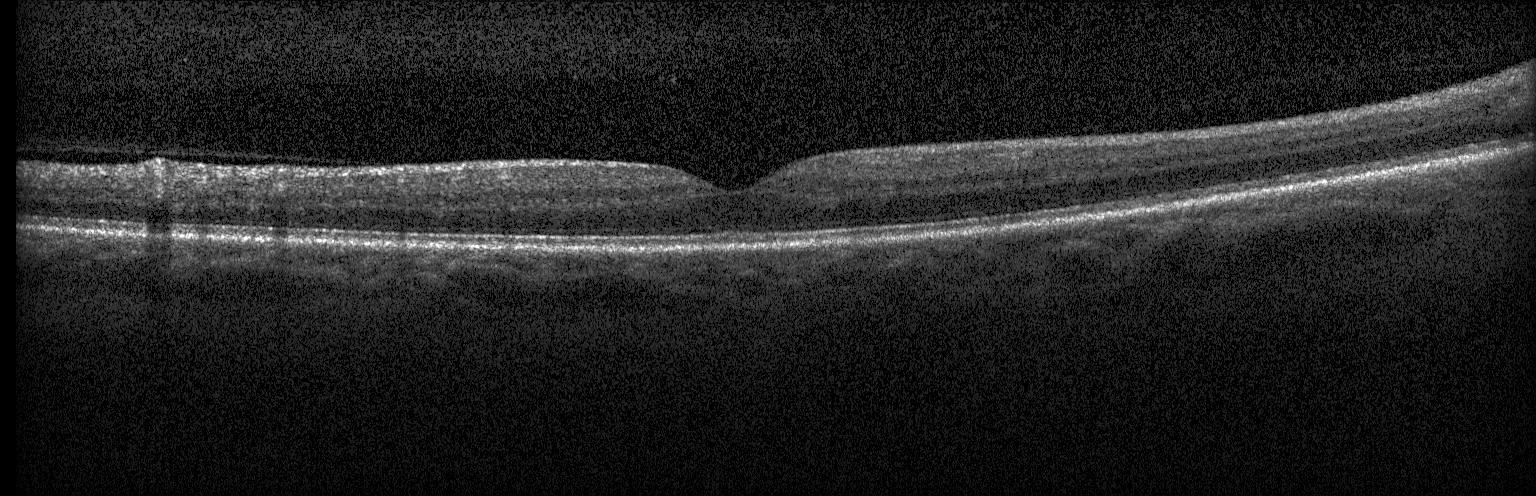 Centered on the fovea, Heidelberg Spectralis, spectral-domain optical coherence tomography, optical coherence tomography scan
Finding: no choroidal neovascularization, diabetic macular edema, or drusen.